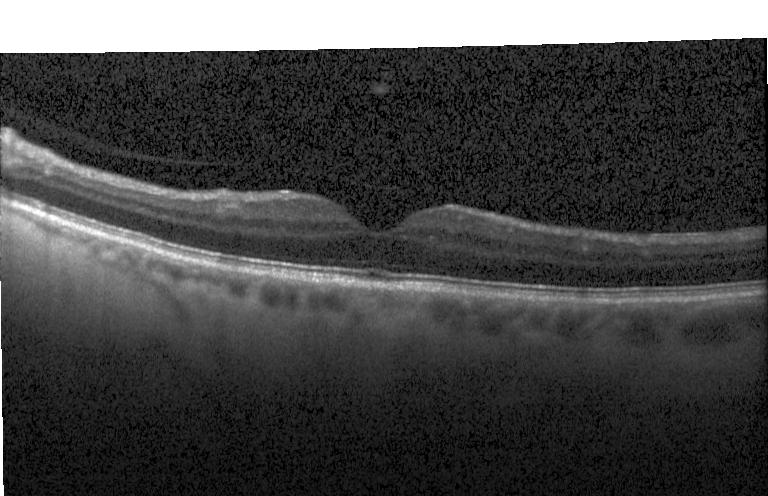
Heidelberg Spectralis · retinal OCT cross-section. The scan shows no CNV, no DME, and no drusen.